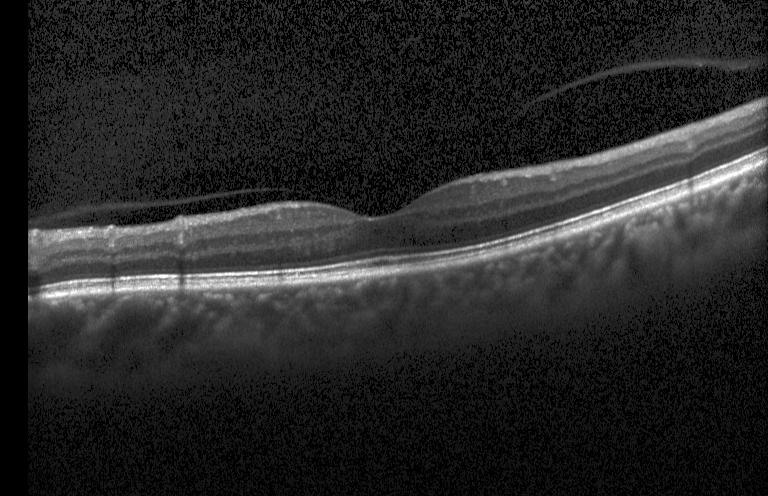 OCT B-scan; Heidelberg Spectralis; macular scan.
No evidence of choroidal neovascularization, diabetic macular edema, or drusen.